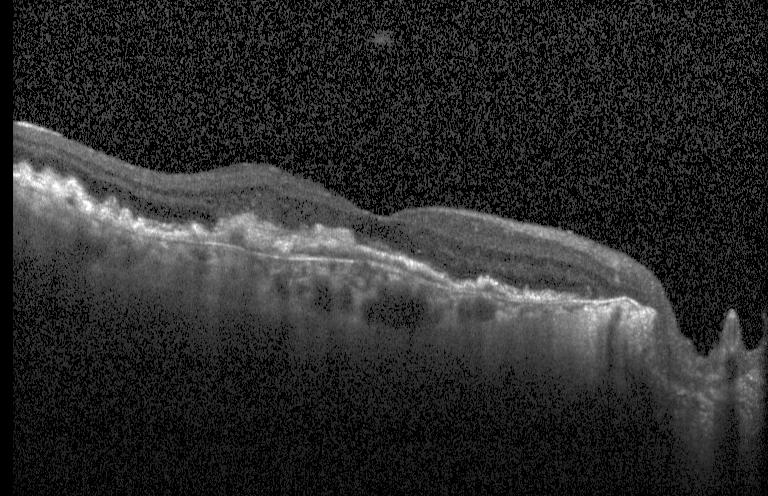
Diagnosis: a choroidal neovascular membrane.